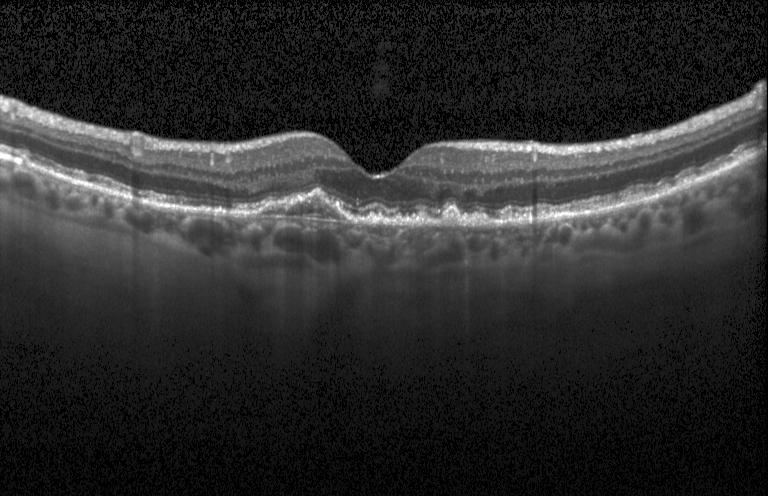
Heidelberg Spectralis; SD-OCT; OCT B-scan
A choroidal neovascular membrane.